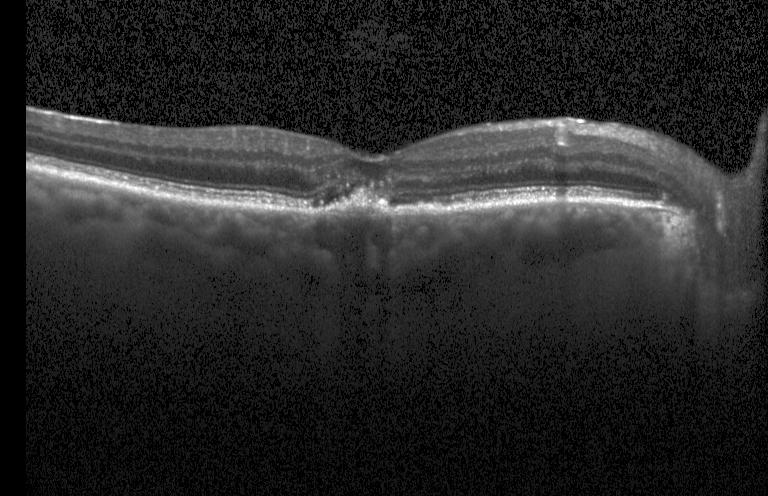
Heidelberg Spectralis, OCT B-scan.
Dx: a choroidal neovascular membrane.